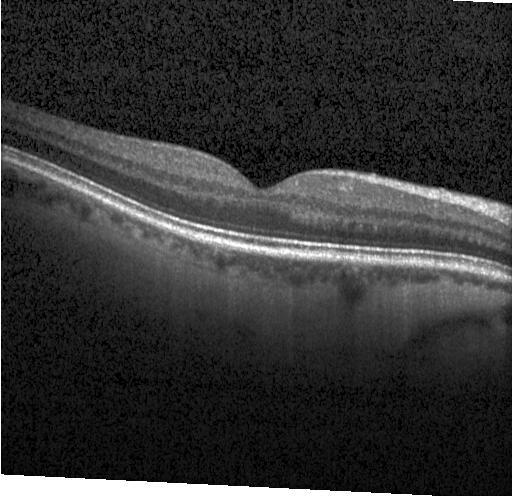

Macular OCT: no choroidal neovascularization, no diabetic macular edema, and no drusen.